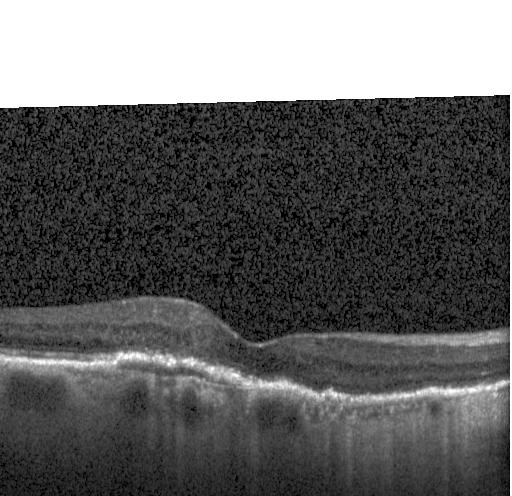

OCT finding: choroidal neovascularization (CNV).